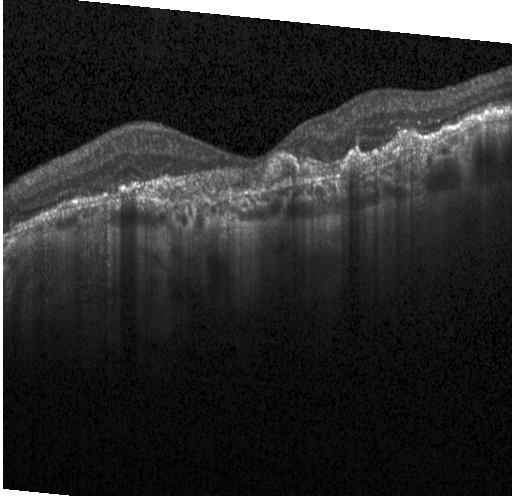
Optical coherence tomography scan. Through the macula. Spectral-domain OCT. Heidelberg Spectralis OCT system — Macular OCT: choroidal neovascularization (CNV).